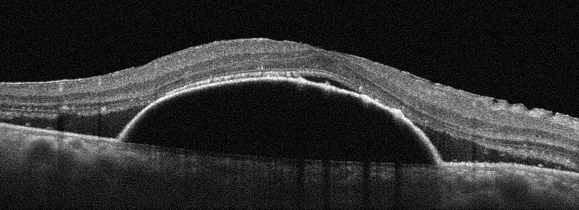
Optical coherence tomography scan, OD.
Assessment: age-related macular degeneration (AMD).